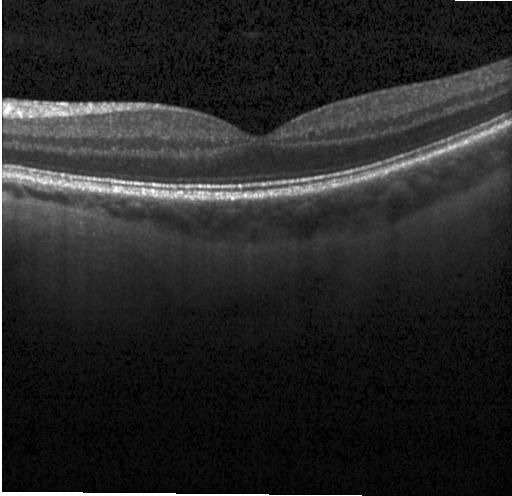
The scan shows no evidence of CNV, DME, or drusen.